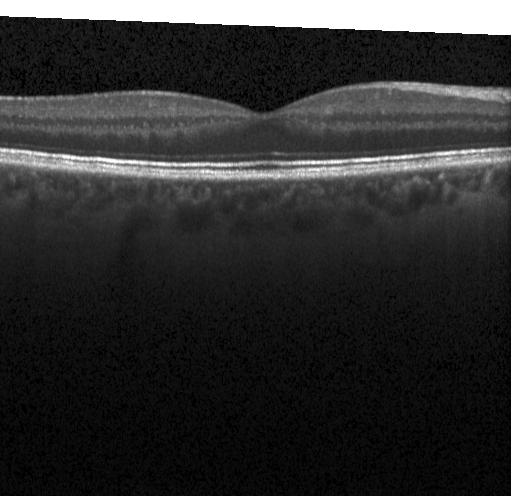

Dx: no choroidal neovascularization, no diabetic macular edema, and no drusen.